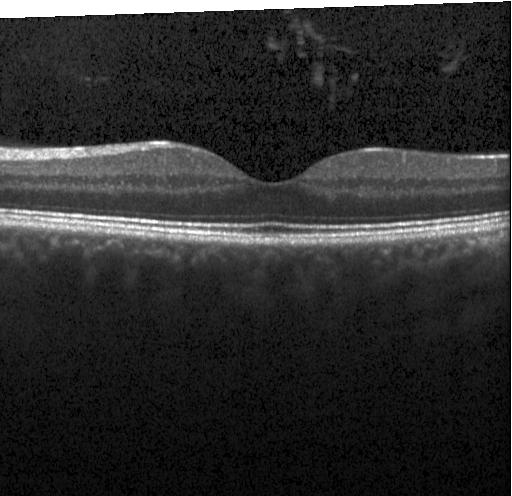 Finding: no choroidal neovascularization, no diabetic macular edema, and no drusen.